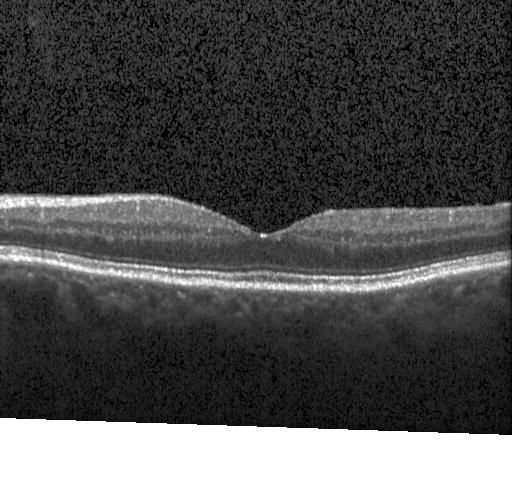
Macular OCT: no evidence of choroidal neovascularization, diabetic macular edema, or drusen.